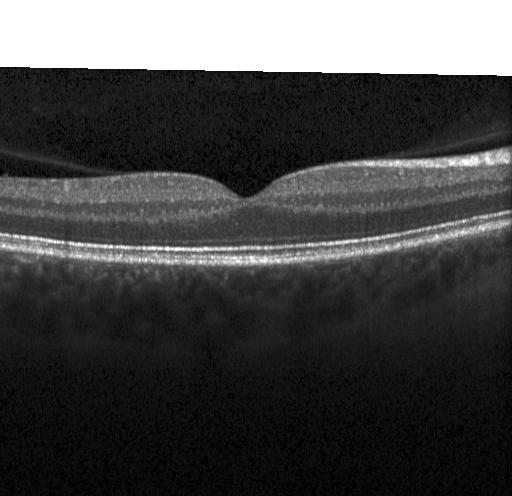

Retinal OCT B-scan — Finding: neither choroidal neovascularization, diabetic macular edema, nor drusen.